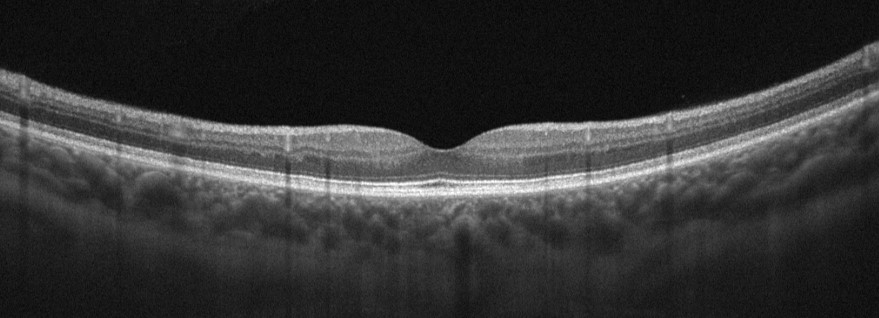
OCT B-scan — Assessment: absence of AMD, DME, ERM, RAO, RVO, and vitreomacular interface disease.